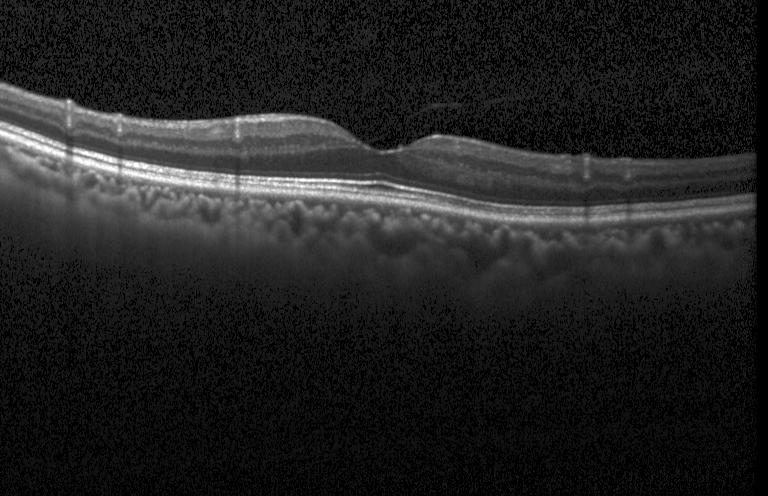

Optical coherence tomography scan, centered on the fovea, spectral-domain OCT, instrument: Heidelberg Spectralis. The scan shows no choroidal neovascularization, no diabetic macular edema, and no drusen.